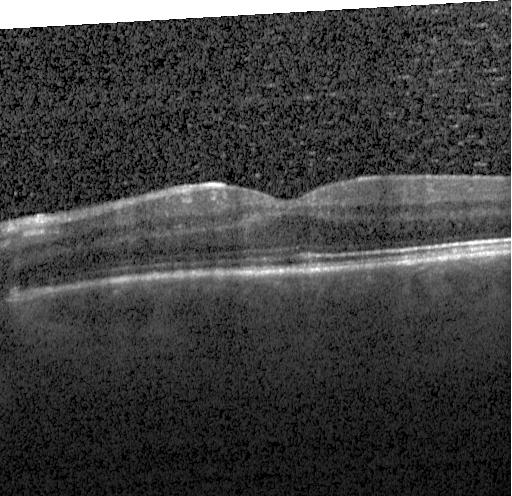

SD-OCT · retinal OCT cross-section · Heidelberg Spectralis OCT system · horizontal scan through the fovea.
Assessment: no choroidal neovascularization, no diabetic macular edema, and no drusen.